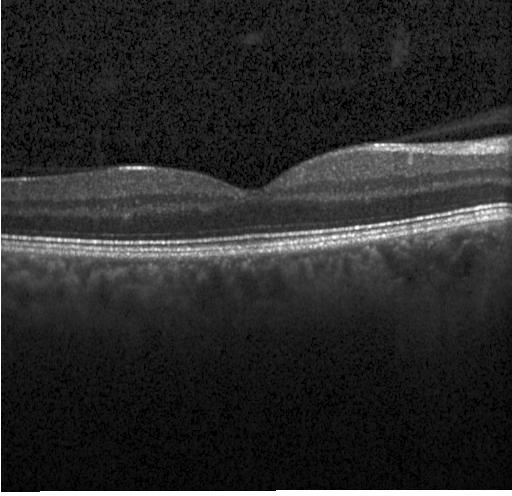 Assessment: no CNV, no DME, and no drusen.